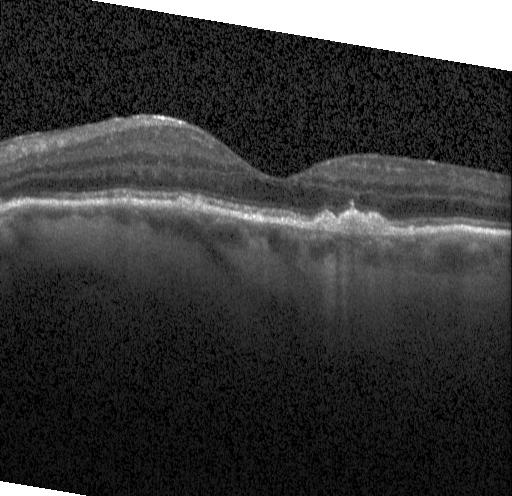

OCT finding: sub-RPE drusenoid deposits.